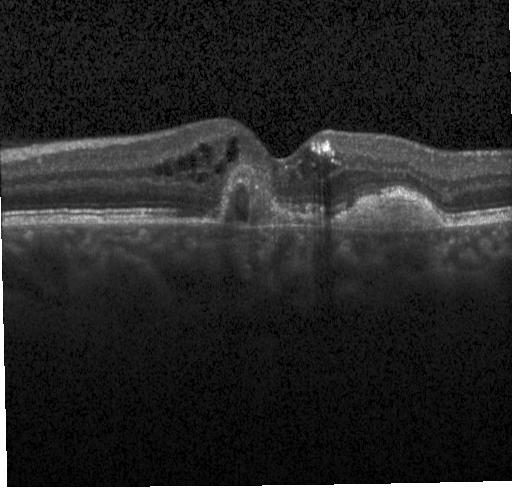 Impression: choroidal neovascularization (CNV).